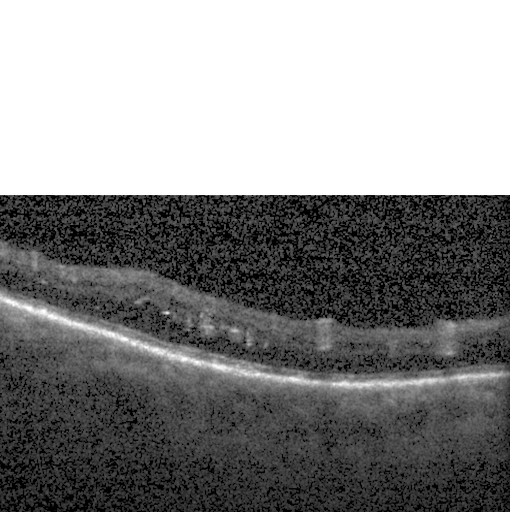
Spectral-domain OCT, retinal OCT cross-section, Heidelberg Spectralis. Diagnosis: diabetic macular edema (DME).